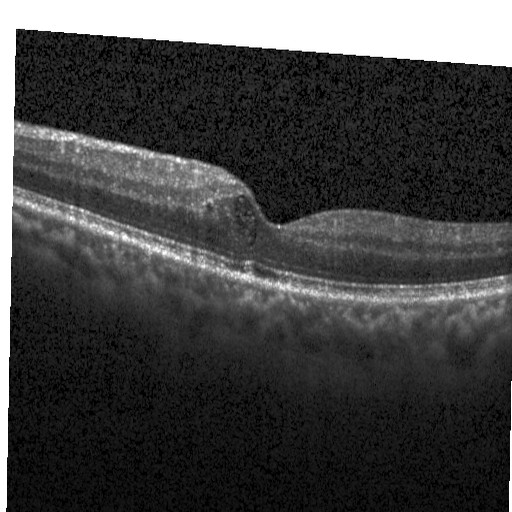 Spectral-domain OCT B-scan: diabetic macular edema (DME).